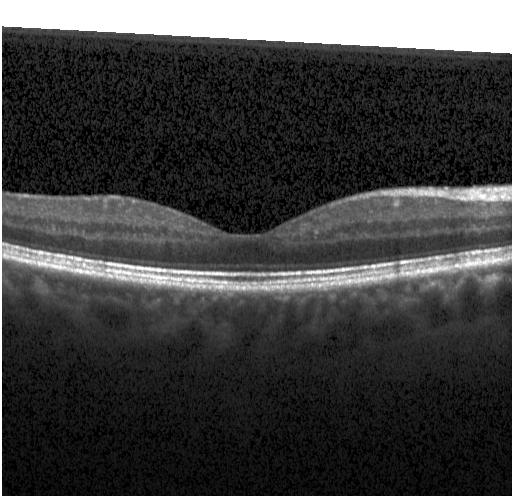
Diagnosis: no evidence of choroidal neovascularization, diabetic macular edema, or drusen.